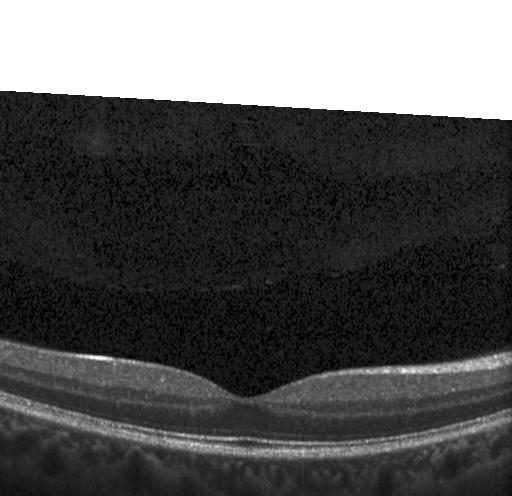
OCT B-scan, centered on the fovea, spectral-domain optical coherence tomography, acquired on a Heidelberg Spectralis — Assessment: no CNV, DME, or drusen.